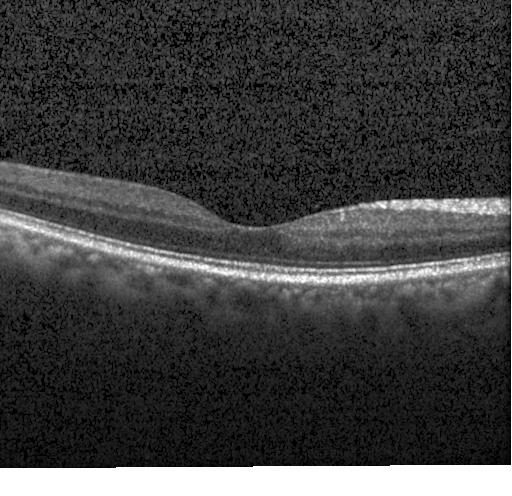
Heidelberg Spectralis. Fovea-centered. Spectral-domain OCT. Retinal OCT cross-section.
Dx: no choroidal neovascularization, no diabetic macular edema, and no drusen.